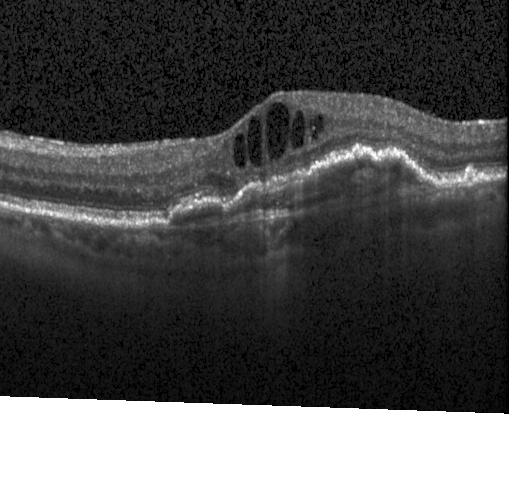

Fovea-centered · instrument: Heidelberg Spectralis · optical coherence tomography scan · spectral-domain optical coherence tomography
Diagnosis: choroidal neovascularization.